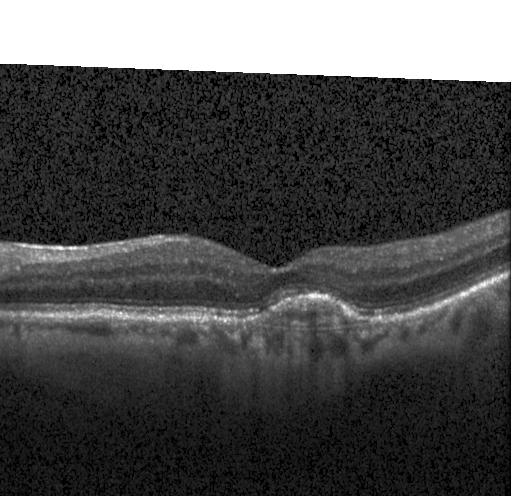

Diagnosis: a choroidal neovascular membrane.